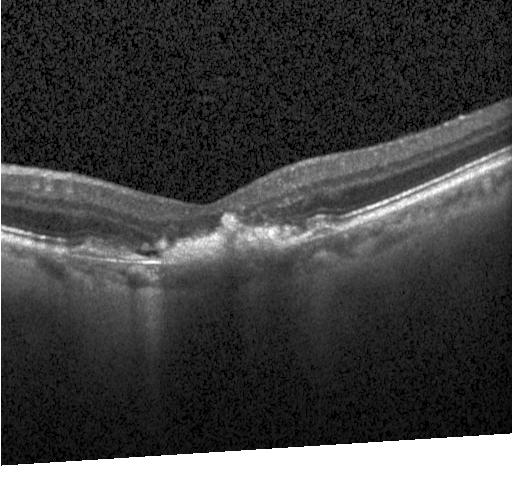

OCT scan showing choroidal neovascularization.